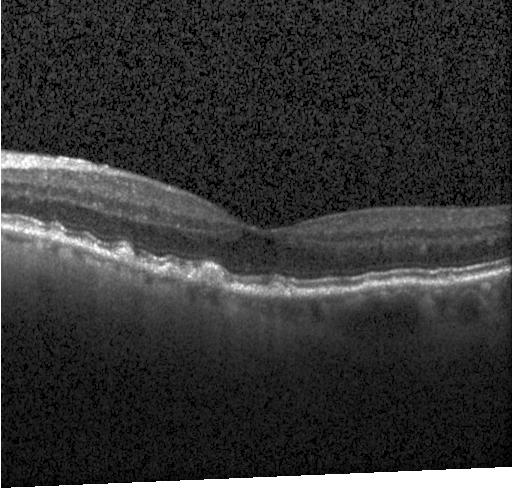
Macular OCT: drusen.